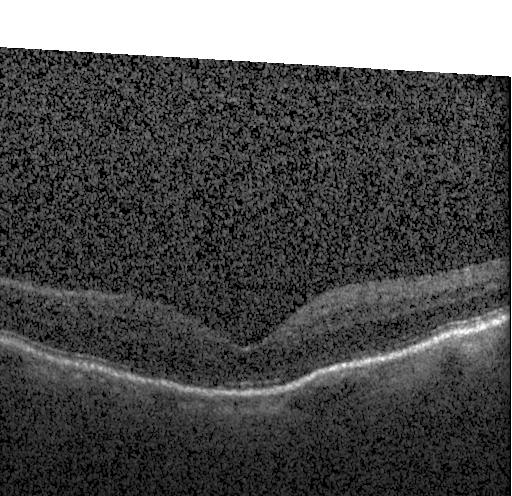
Assessment: neither choroidal neovascularization, diabetic macular edema, nor drusen.